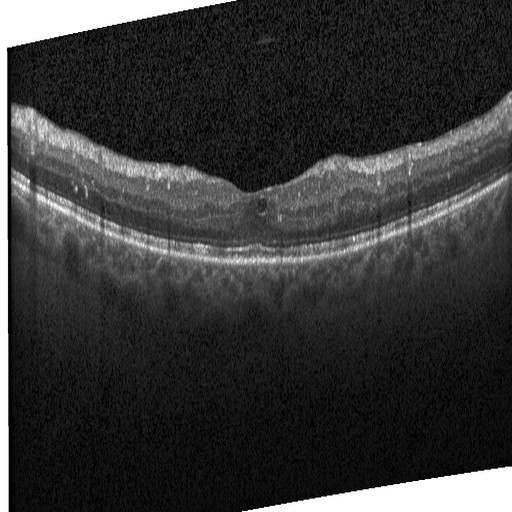
Heidelberg Spectralis; optical coherence tomography scan; fovea-centered. This B-scan demonstrates diabetic macular edema (DME).